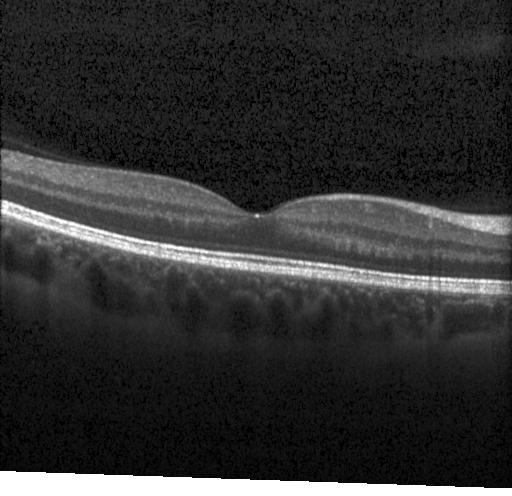
Fovea-centered; OCT B-scan; Heidelberg Spectralis OCT system.
OCT finding: no CNV, no DME, and no drusen.